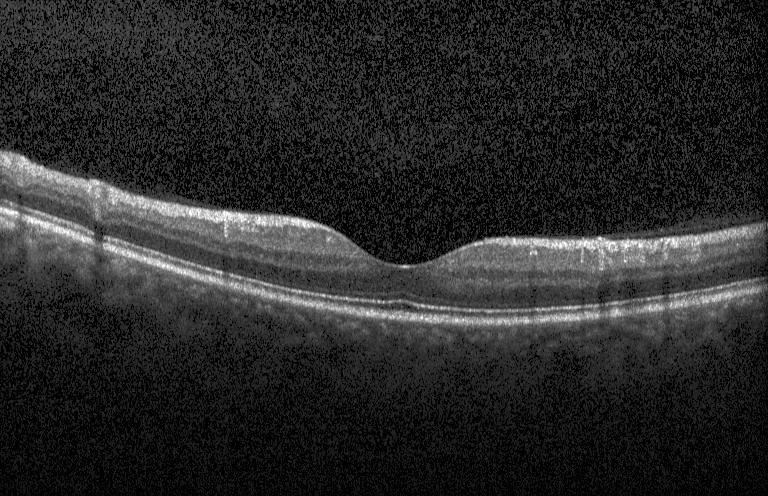

Heidelberg Spectralis OCT system; SD-OCT; fovea-centered; OCT B-scan — This B-scan demonstrates neither choroidal neovascularization, diabetic macular edema, nor drusen.